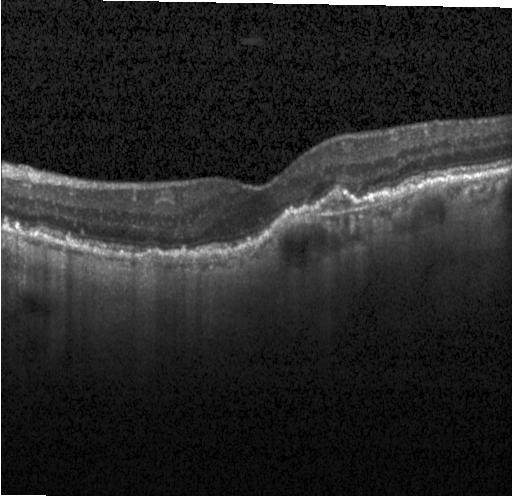

Dx: choroidal neovascularization (CNV).